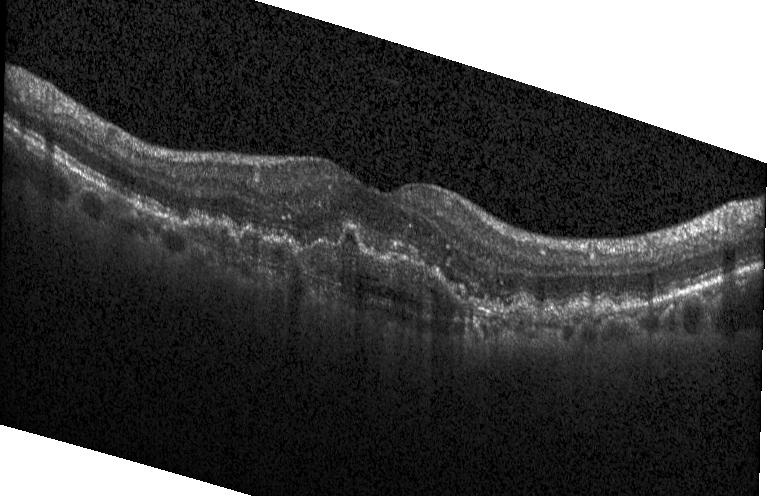
This B-scan demonstrates CNV.